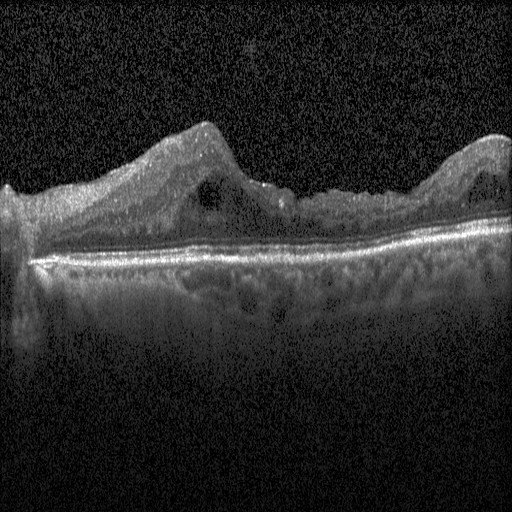
Diagnosis: DME.